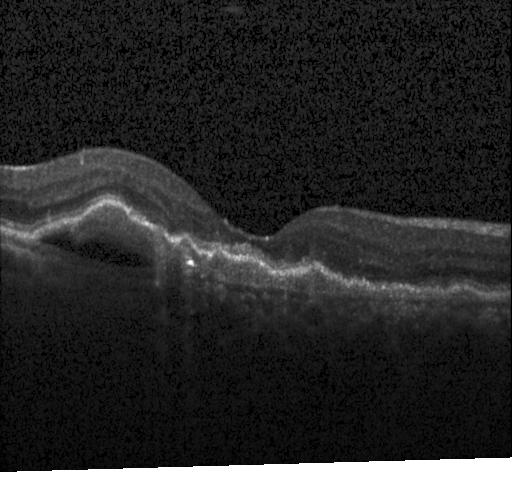 Retinal OCT B-scan — Finding: choroidal neovascularization.